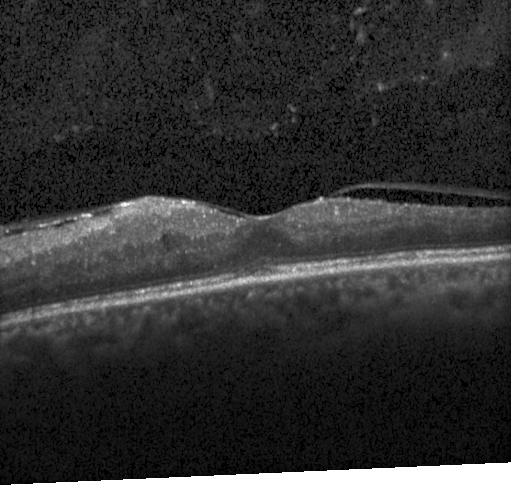

Centered on the fovea · spectral-domain OCT · retinal OCT B-scan · Heidelberg Spectralis OCT system.
Dx: diabetic macular edema.